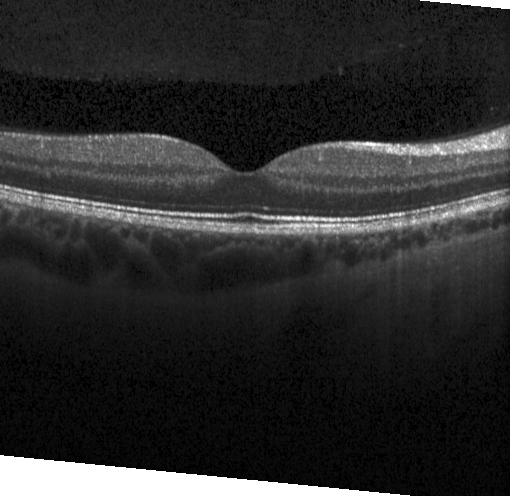
OCT line scan · Heidelberg Spectralis OCT system · macular scan
The scan shows no choroidal neovascularization, diabetic macular edema, or drusen.